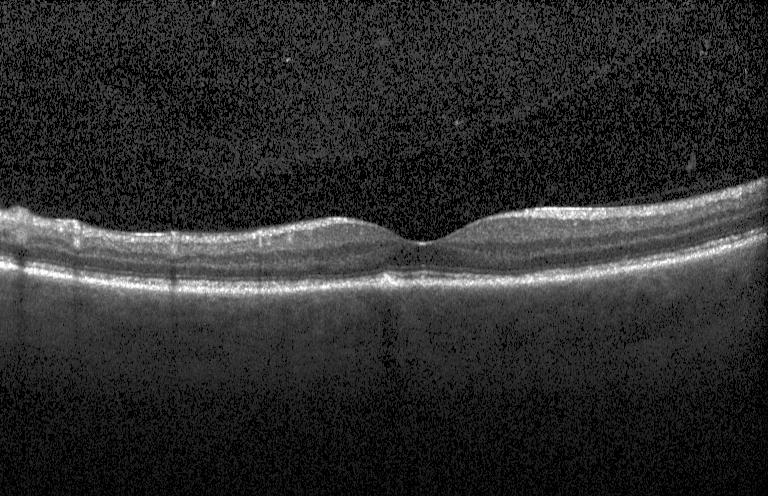 Dx: multiple drusen.